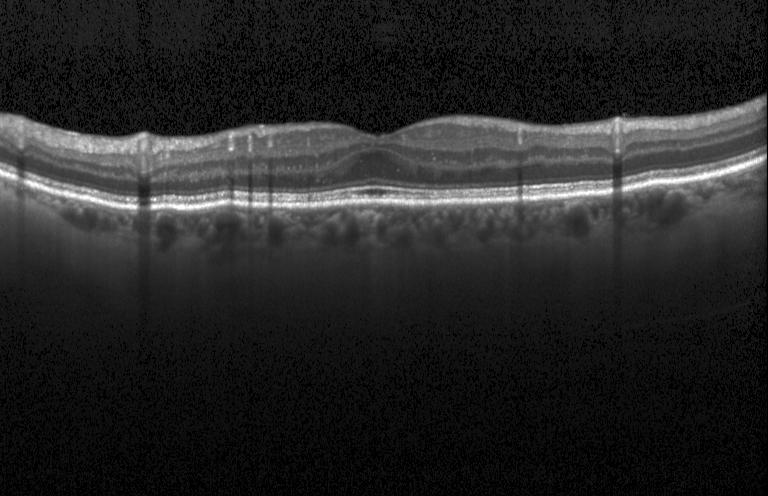
Impression: no choroidal neovascularization, no diabetic macular edema, and no drusen.